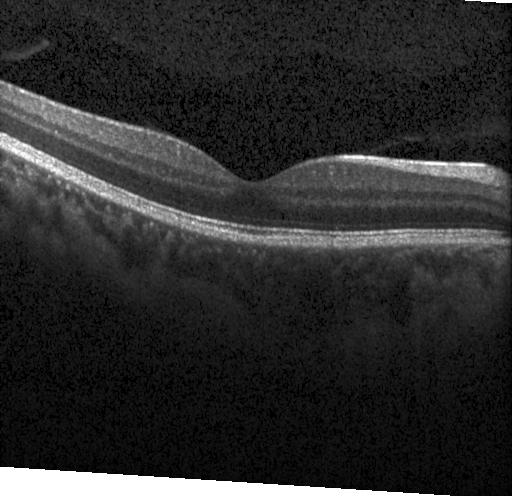 Retinal OCT cross-section; Heidelberg Spectralis.
Assessment: no CNV, no DME, and no drusen.